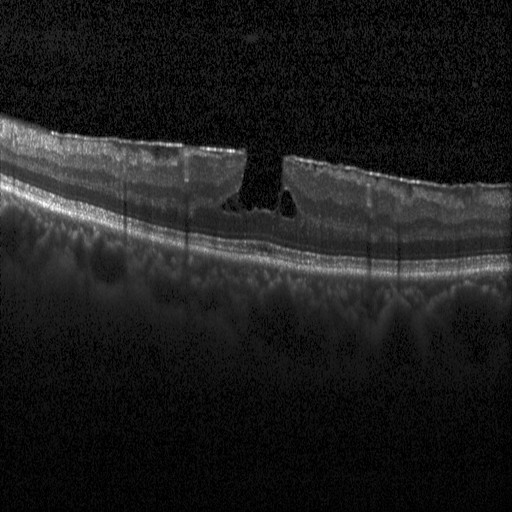 DME.